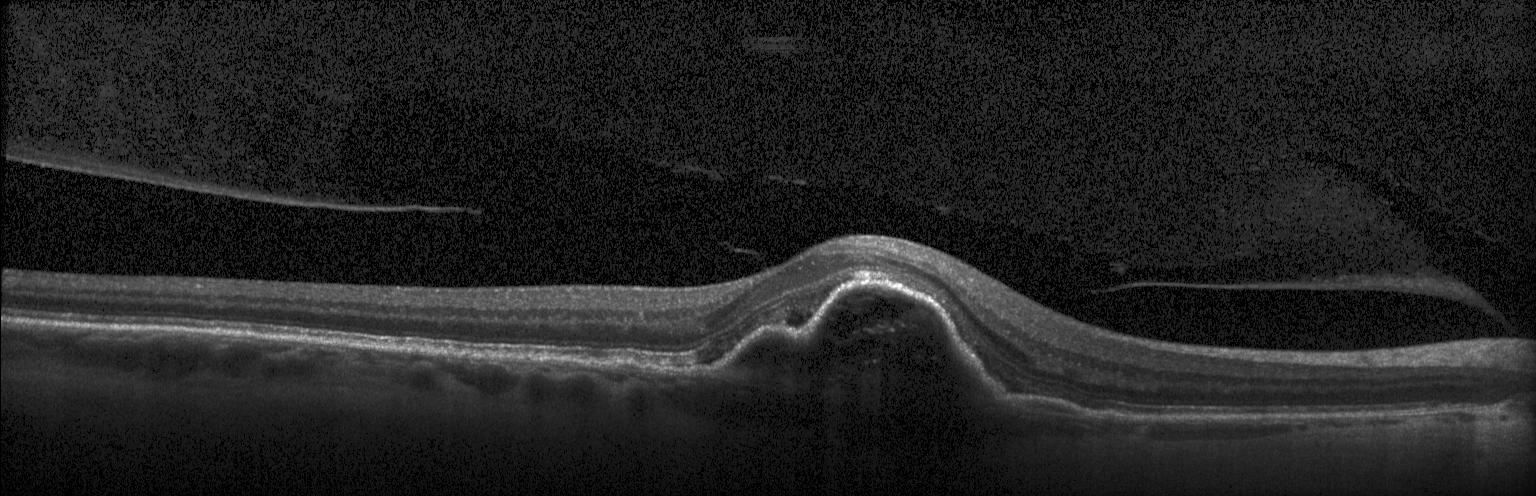
Optical coherence tomography scan
Diagnosis: a choroidal neovascular membrane.